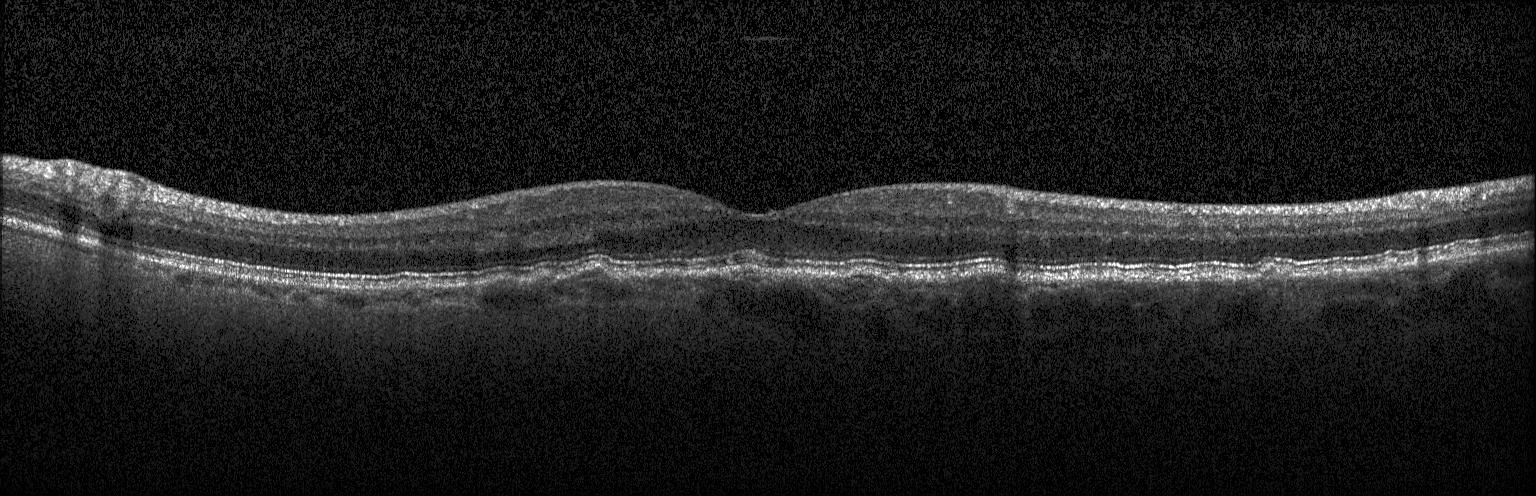 Finding: sub-RPE drusenoid deposits.